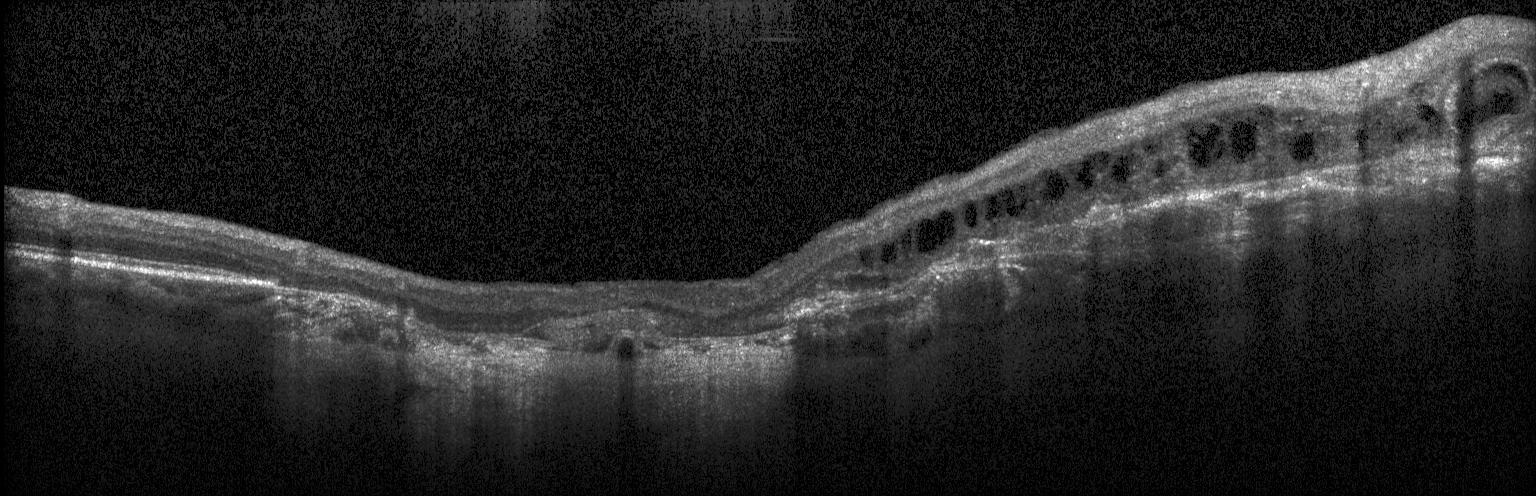 Retinal OCT cross-section
Finding: a choroidal neovascular membrane.